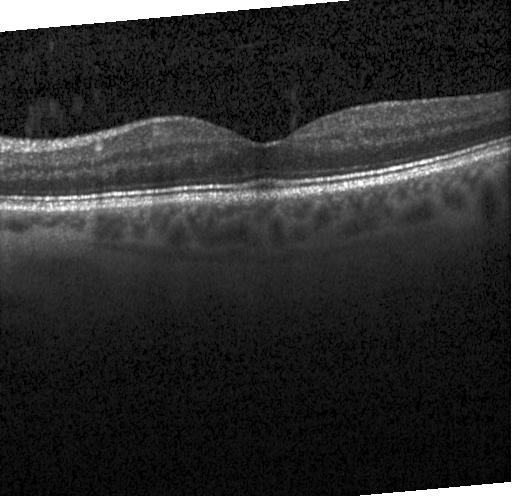
Horizontal scan through the fovea. Spectral-domain OCT. Instrument: Heidelberg Spectralis. Retinal OCT B-scan. Macular OCT: no choroidal neovascularization, diabetic macular edema, or drusen.